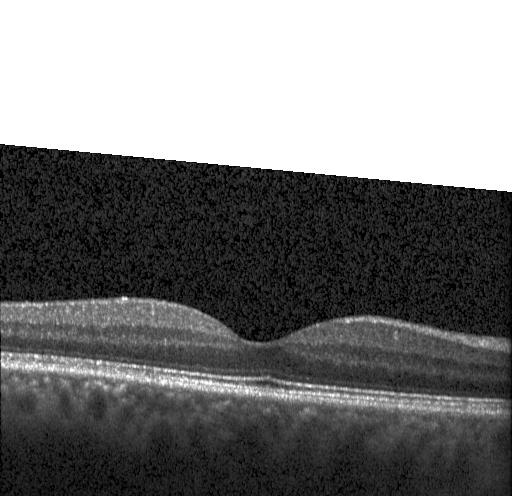
Finding: no choroidal neovascularization, diabetic macular edema, or drusen.